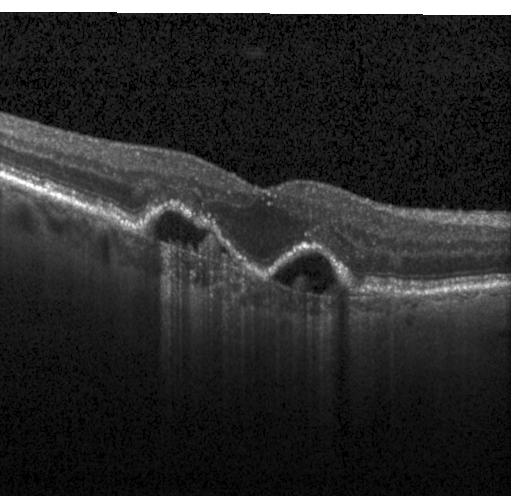

Macular scan. Optical coherence tomography scan. Instrument: Heidelberg Spectralis. Spectral-domain optical coherence tomography — Impression: CNV.